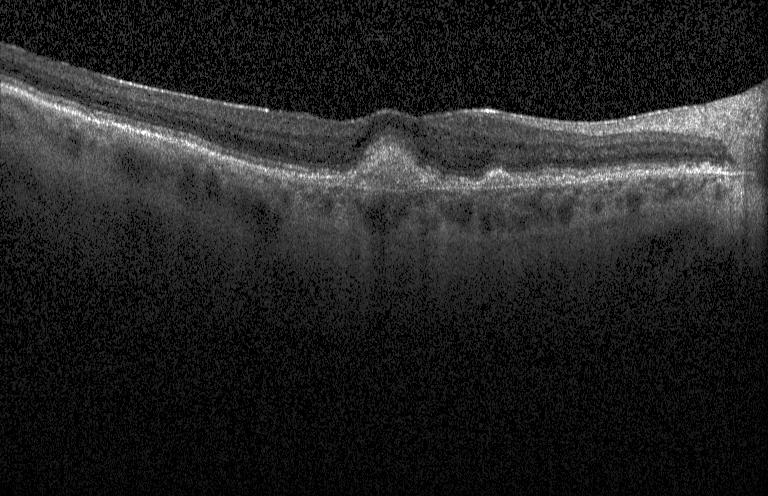
Horizontal scan through the fovea, retinal OCT cross-section, Heidelberg Spectralis
Impression: a choroidal neovascular membrane.